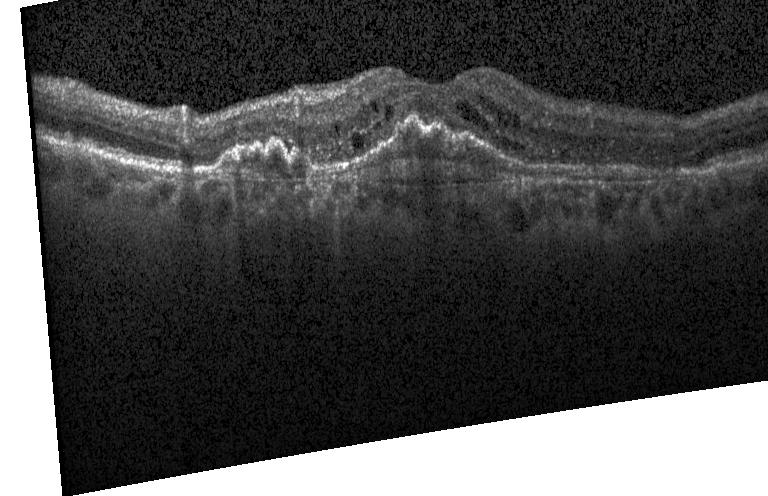

Assessment: a choroidal neovascular membrane.